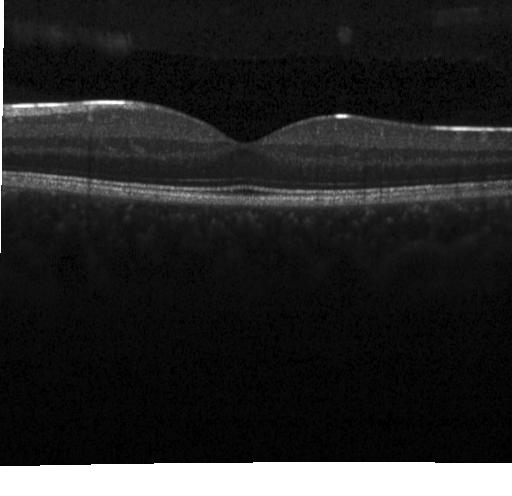
Spectral-domain OCT. OCT B-scan.
The scan shows no evidence of choroidal neovascularization, diabetic macular edema, or drusen.